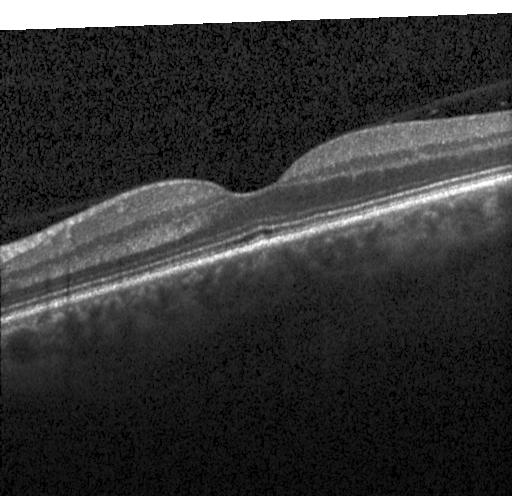
Impression: neither choroidal neovascularization, diabetic macular edema, nor drusen.